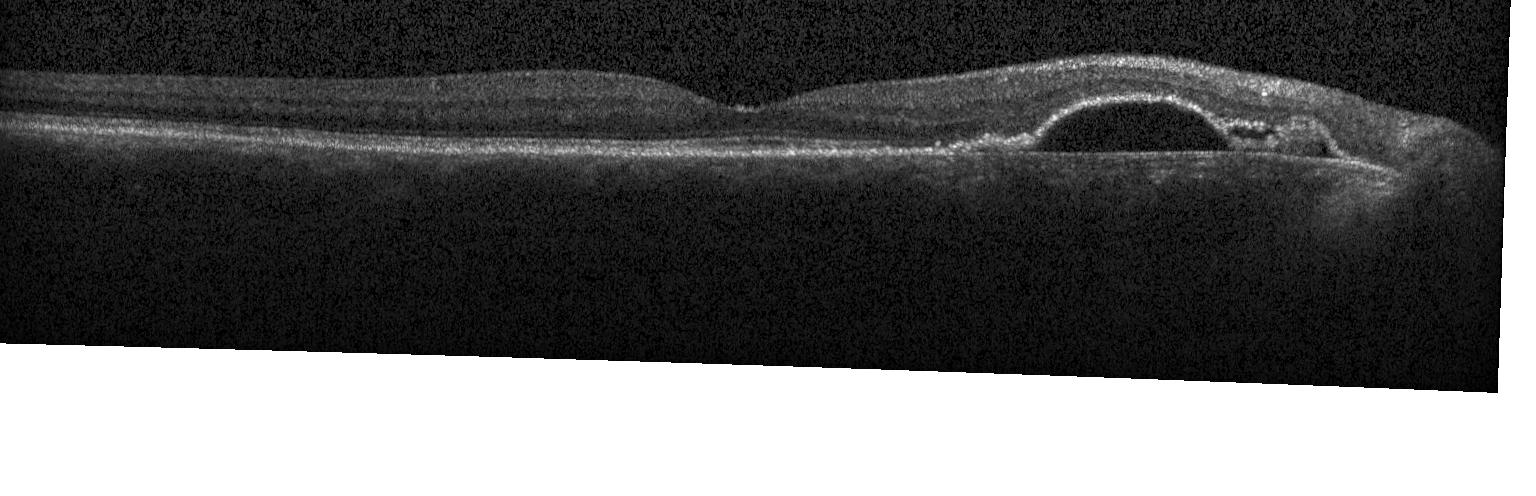 Impression: choroidal neovascularization.